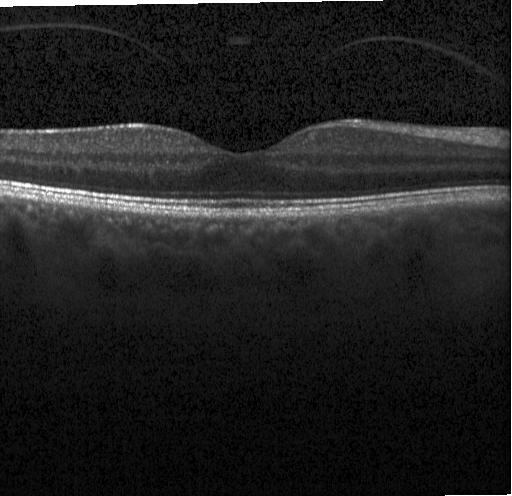

Heidelberg Spectralis OCT system, OCT line scan
Neither choroidal neovascularization, diabetic macular edema, nor drusen.